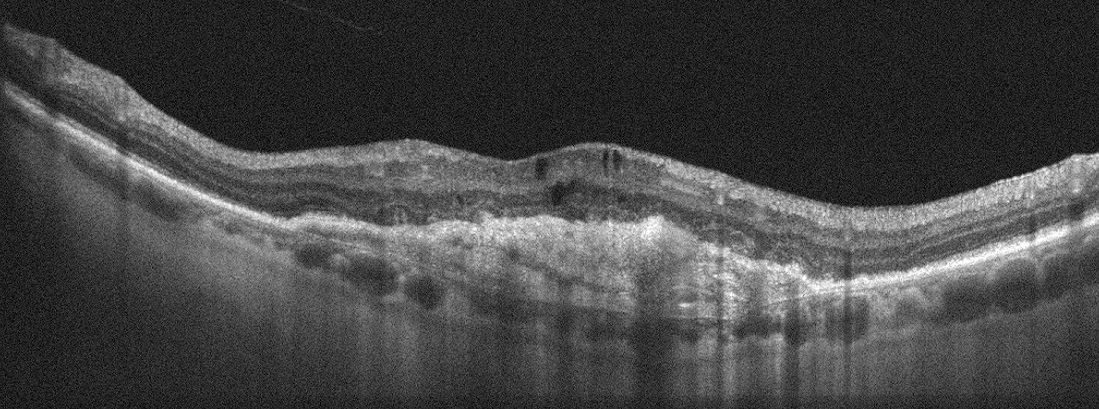

Retinal OCT cross-section, through the macula, instrument: Optovue Avanti RTVue XR — This B-scan demonstrates AMD.